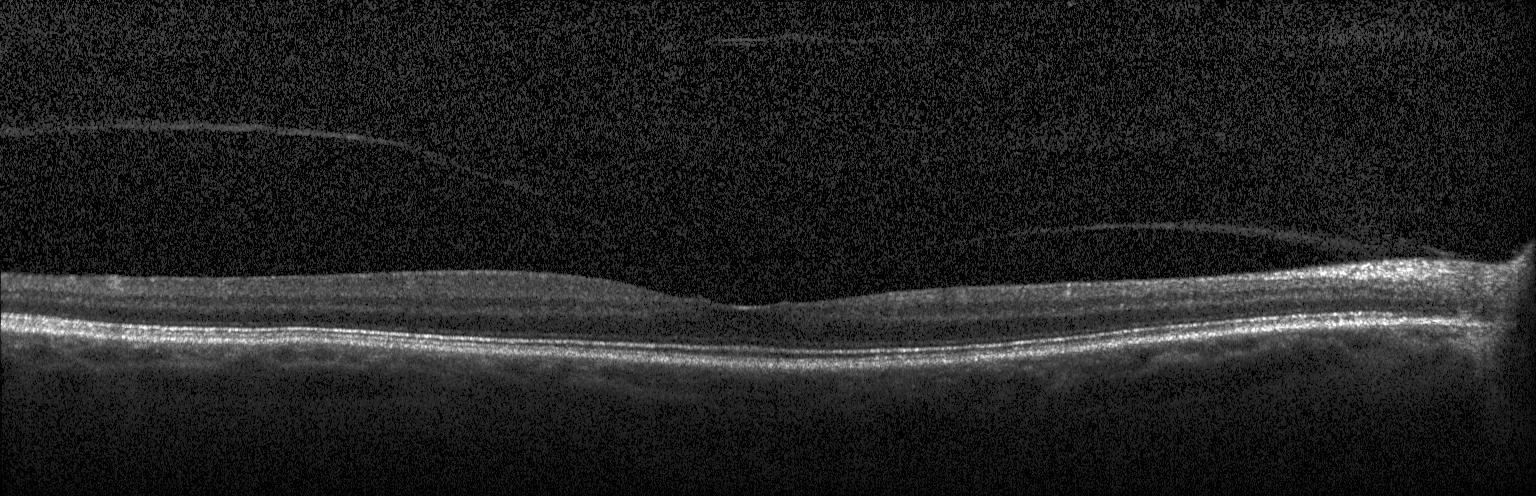

Spectral-domain OCT, OCT line scan, acquired on a Heidelberg Spectralis, fovea-centered. Diagnosis: neither choroidal neovascularization, diabetic macular edema, nor drusen.